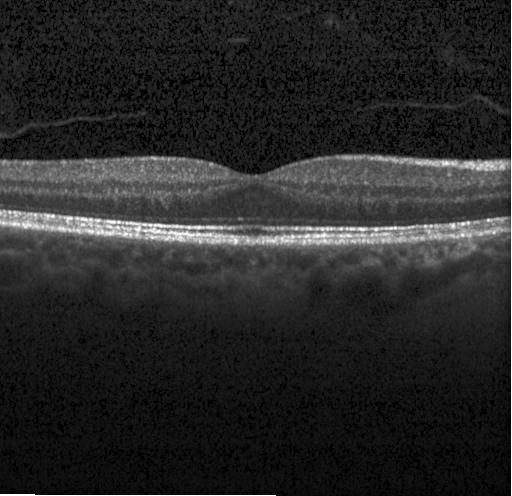
Spectral-domain optical coherence tomography; optical coherence tomography B-scan; fovea-centered; Heidelberg Spectralis.
Impression: no choroidal neovascularization, no diabetic macular edema, and no drusen.